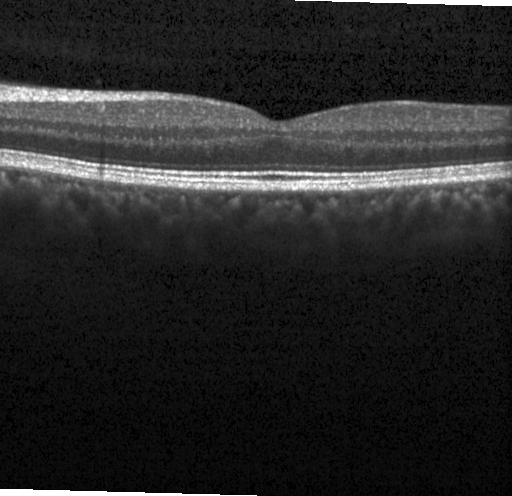

Through the macula. Optical coherence tomography B-scan. SD-OCT. Instrument: Heidelberg Spectralis.
Impression: no choroidal neovascularization, no diabetic macular edema, and no drusen.